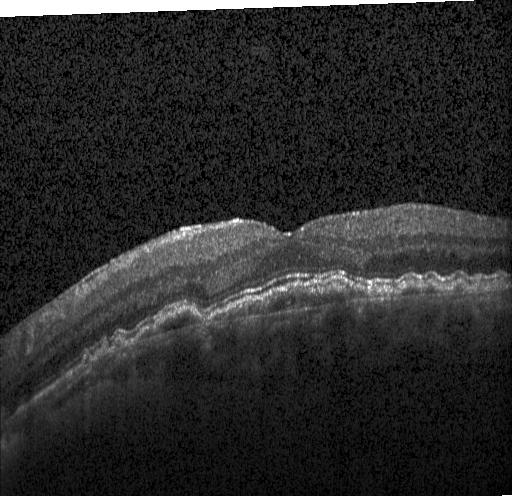

Diagnosis: CNV.